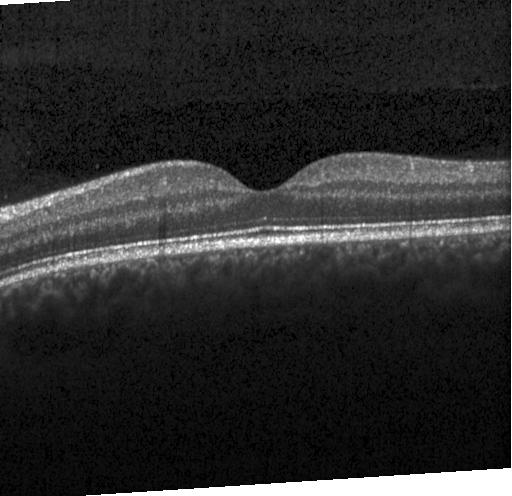

Retinal OCT cross-section — Diagnosis: neither CNV, DME, nor drusen.